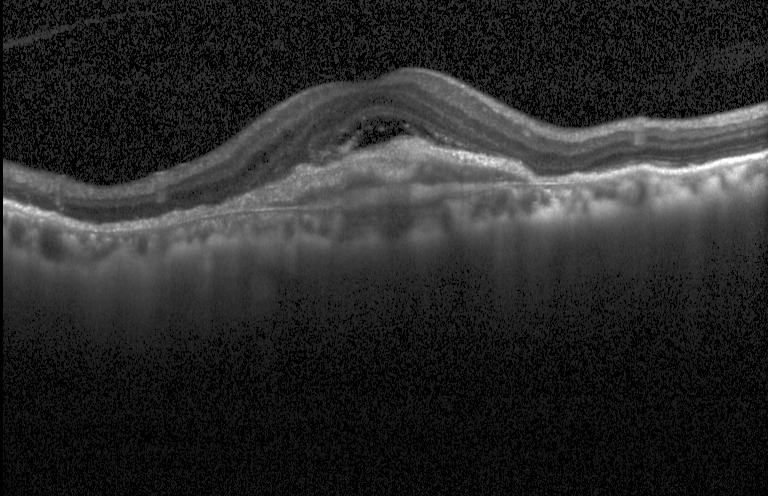

OCT scan showing choroidal neovascularization.